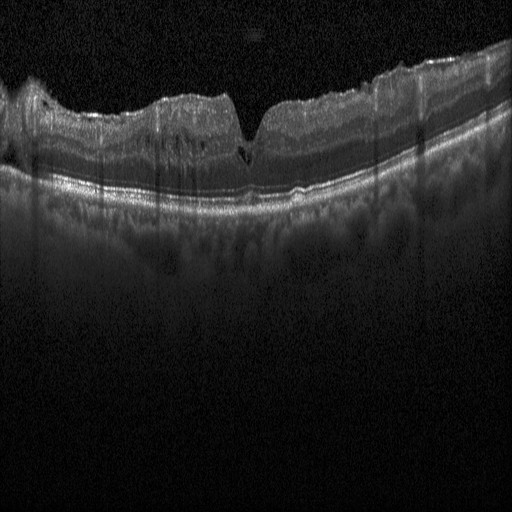

Retinal OCT B-scan; Heidelberg Spectralis OCT system; SD-OCT
This B-scan demonstrates diabetic macular edema.